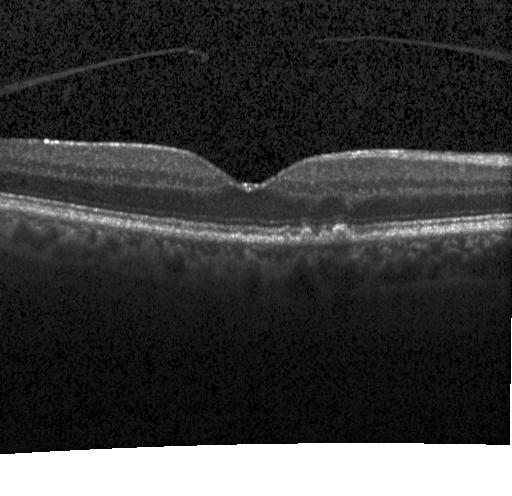
Macular OCT: multiple drusen.